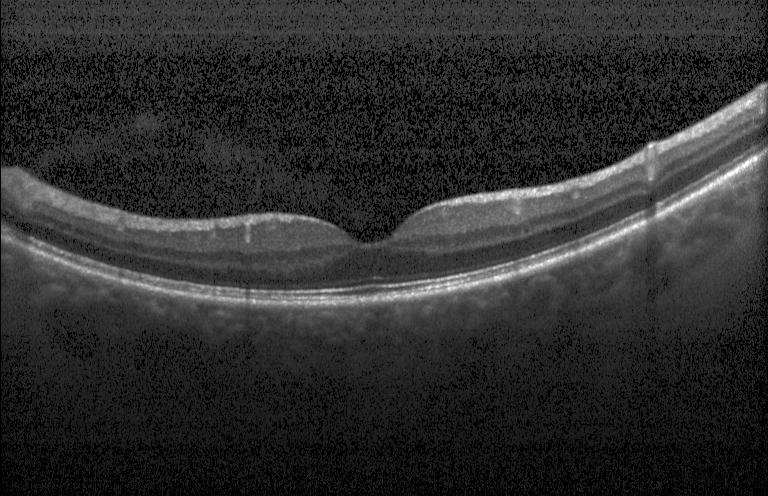

Horizontal scan through the fovea · SD-OCT · instrument: Heidelberg Spectralis · retinal OCT cross-section — OCT finding: no choroidal neovascularization, diabetic macular edema, or drusen.